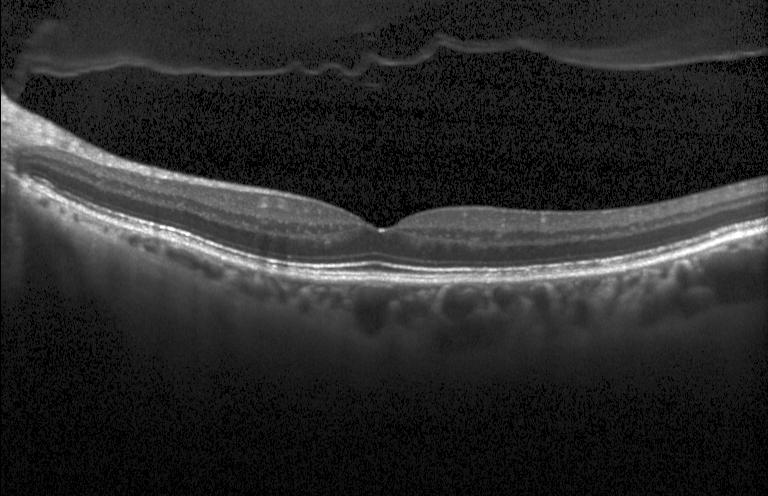 Through the macula; SD-OCT; retinal OCT cross-section; Heidelberg Spectralis.
Finding: neither choroidal neovascularization, diabetic macular edema, nor drusen.